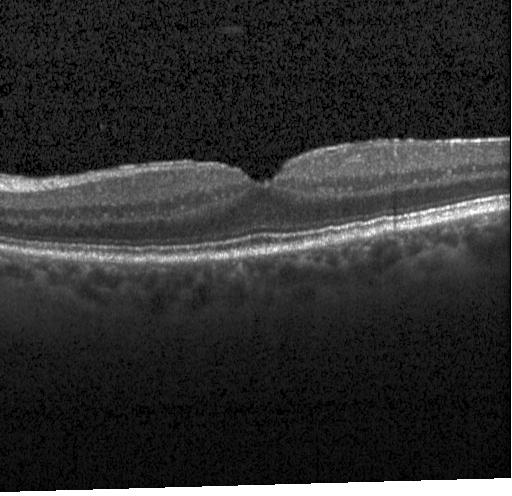
Optical coherence tomography scan; fovea-centered; instrument: Heidelberg Spectralis; spectral-domain OCT
The scan shows neither choroidal neovascularization, diabetic macular edema, nor drusen.